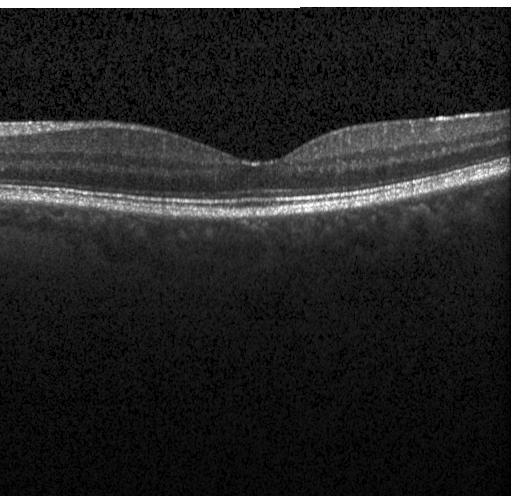 Diagnosis: neither choroidal neovascularization, diabetic macular edema, nor drusen.